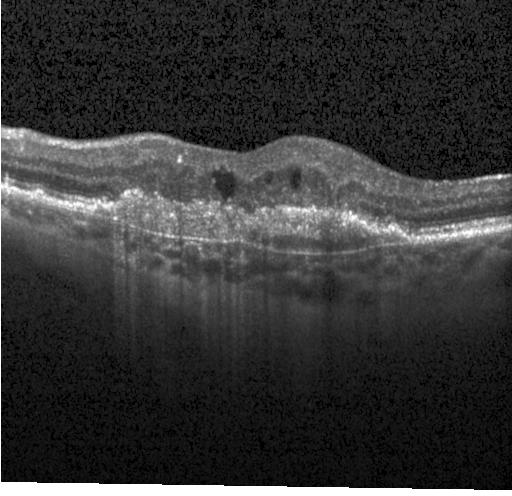 OCT finding: choroidal neovascularization.